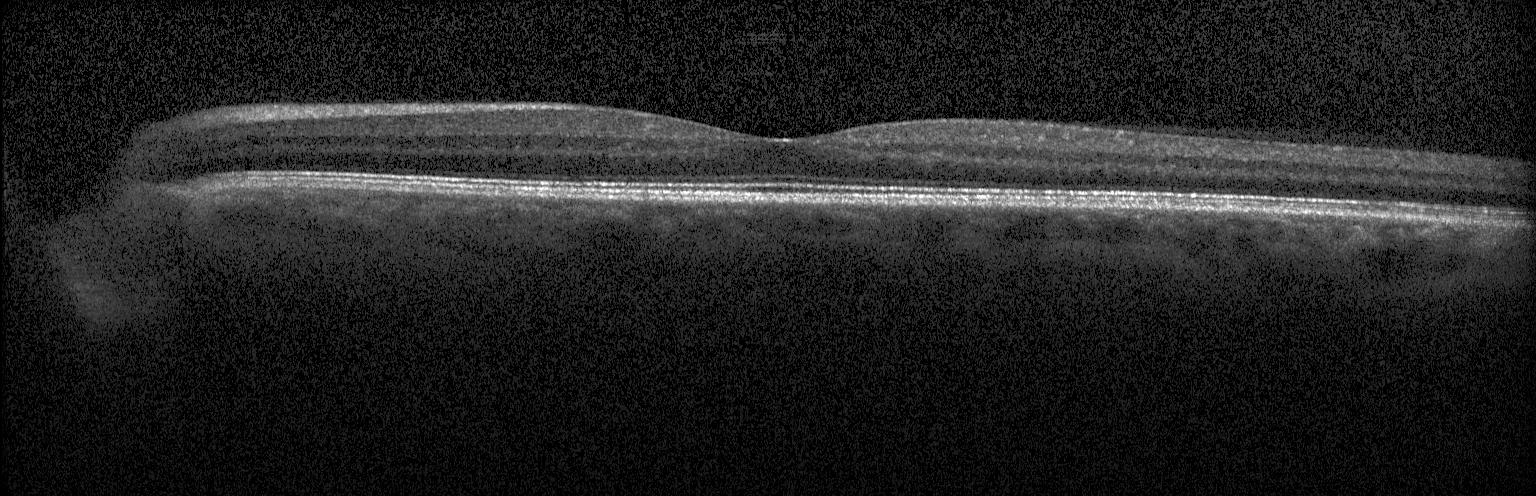 Spectral-domain optical coherence tomography. Optical coherence tomography scan — This B-scan demonstrates no choroidal neovascularization, diabetic macular edema, or drusen.